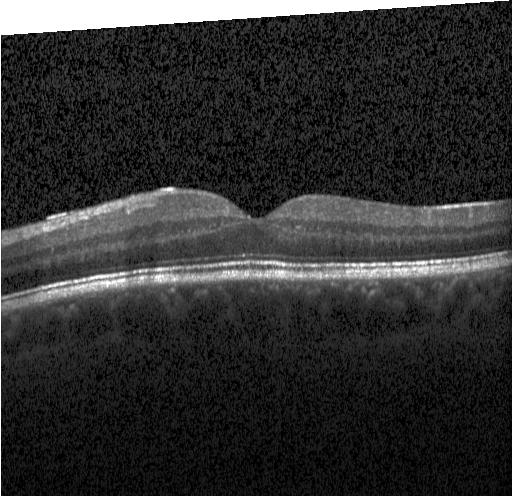
Impression: no CNV, DME, or drusen.